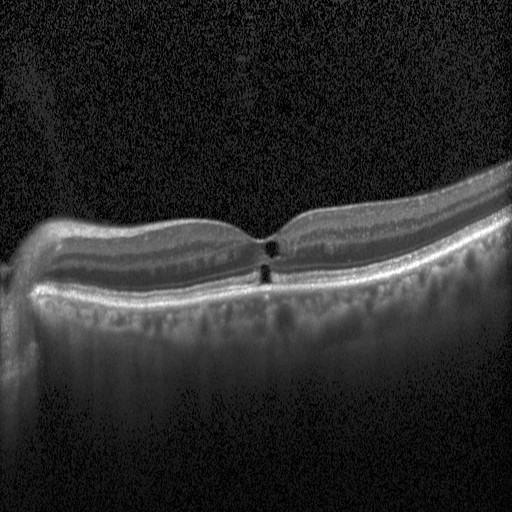
Instrument: Heidelberg Spectralis · retinal OCT B-scan.
Diabetic macular edema.